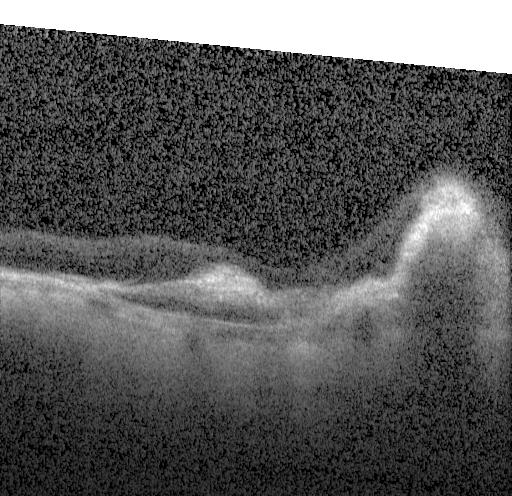
Spectral-domain OCT, optical coherence tomography B-scan — Diagnosis: CNV.